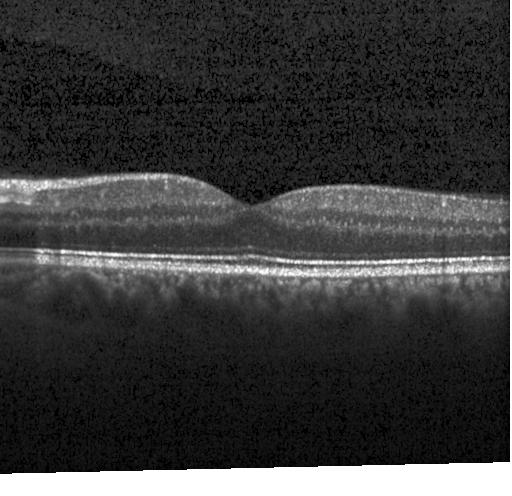
Optical coherence tomography scan.
The scan shows no evidence of choroidal neovascularization, diabetic macular edema, or drusen.